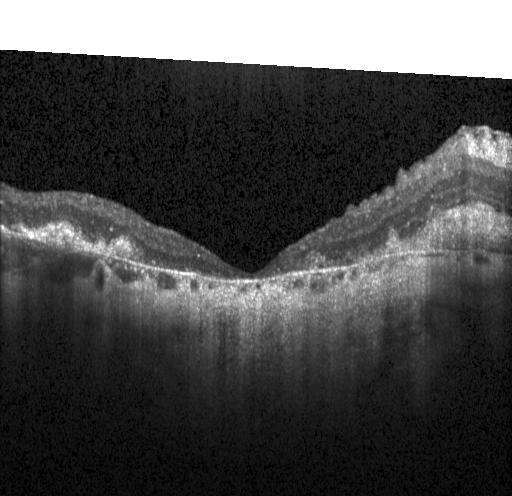

Instrument: Heidelberg Spectralis · OCT B-scan · centered on the fovea · spectral-domain OCT
OCT finding: a choroidal neovascular membrane.